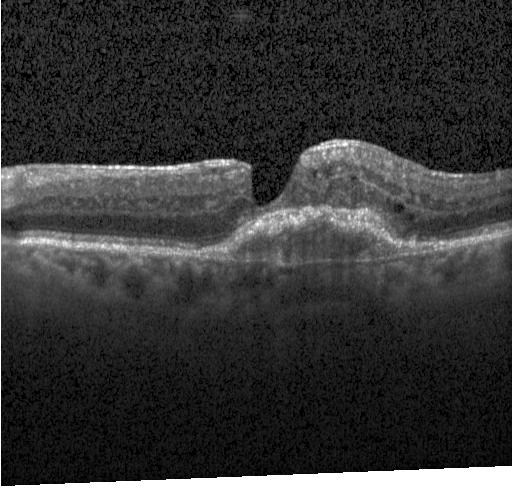

Heidelberg Spectralis. Spectral-domain optical coherence tomography. OCT B-scan
Impression: choroidal neovascularization.